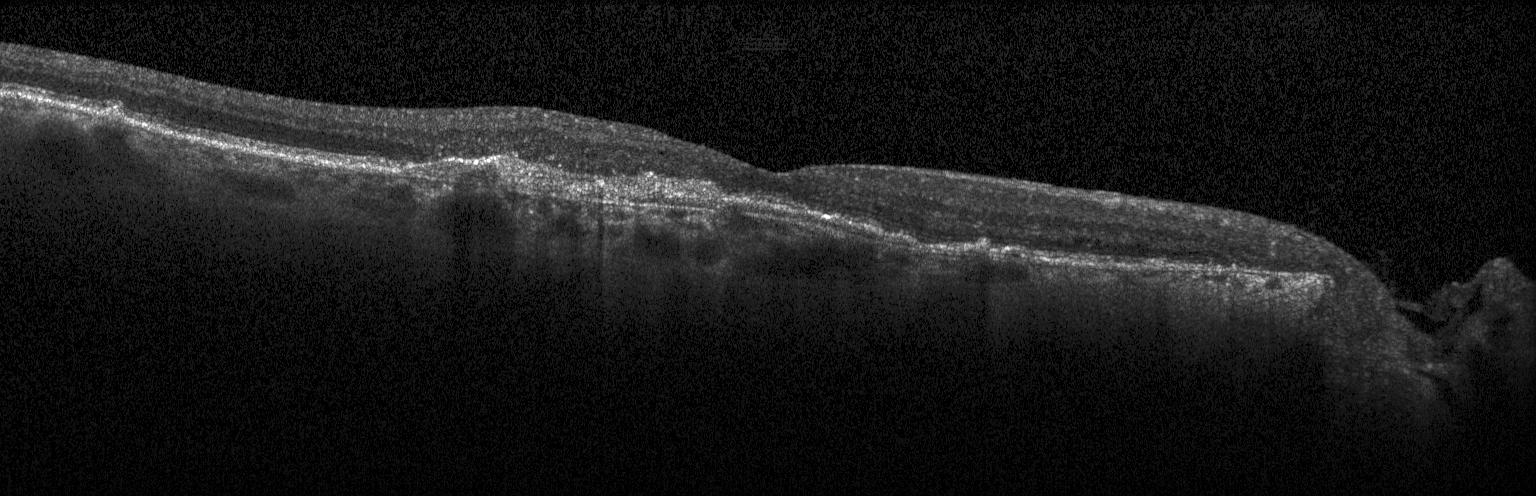

OCT scan showing a choroidal neovascular membrane.